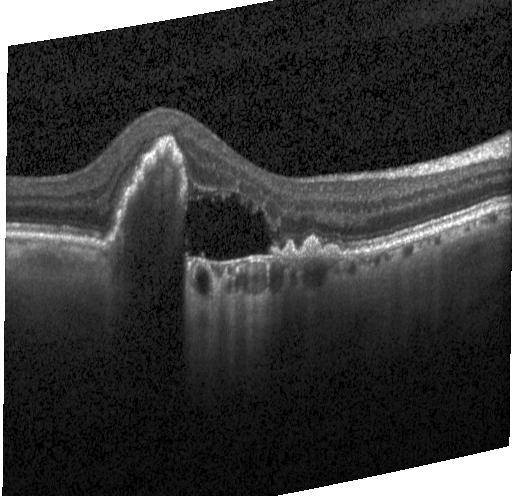 Spectral-domain OCT B-scan: CNV.